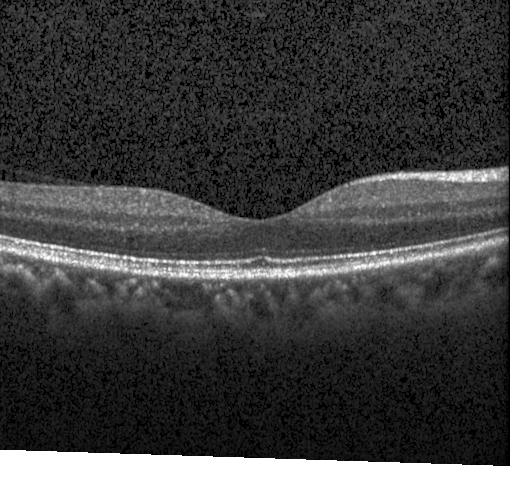
Finding: no CNV, DME, or drusen.